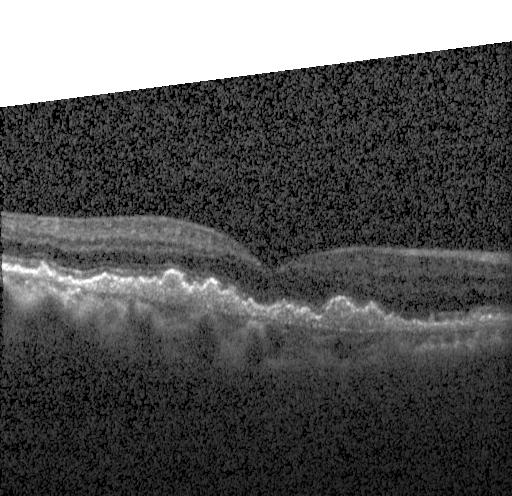

OCT finding: choroidal neovascularization (CNV).